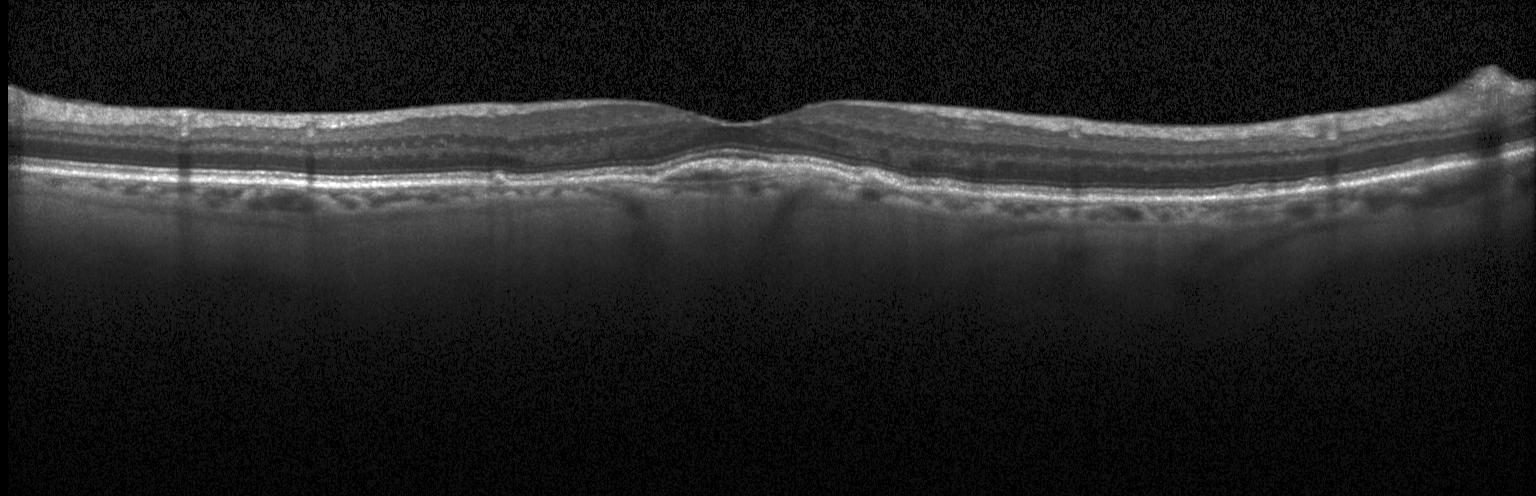 Through the macula, spectral-domain optical coherence tomography, optical coherence tomography scan, Heidelberg Spectralis OCT system
Assessment: CNV.